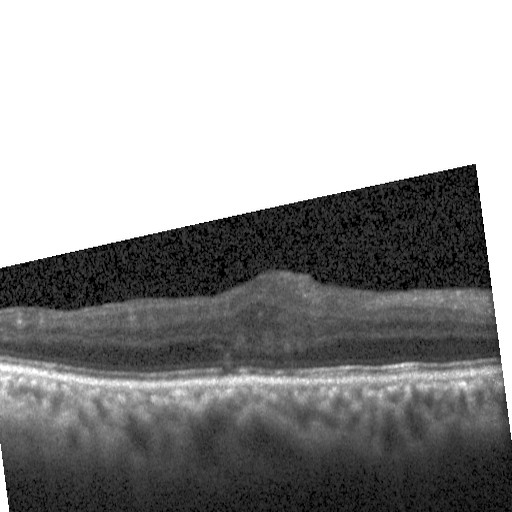
Instrument: Heidelberg Spectralis · retinal OCT cross-section · macular scan · spectral-domain optical coherence tomography. Diabetic macular edema.